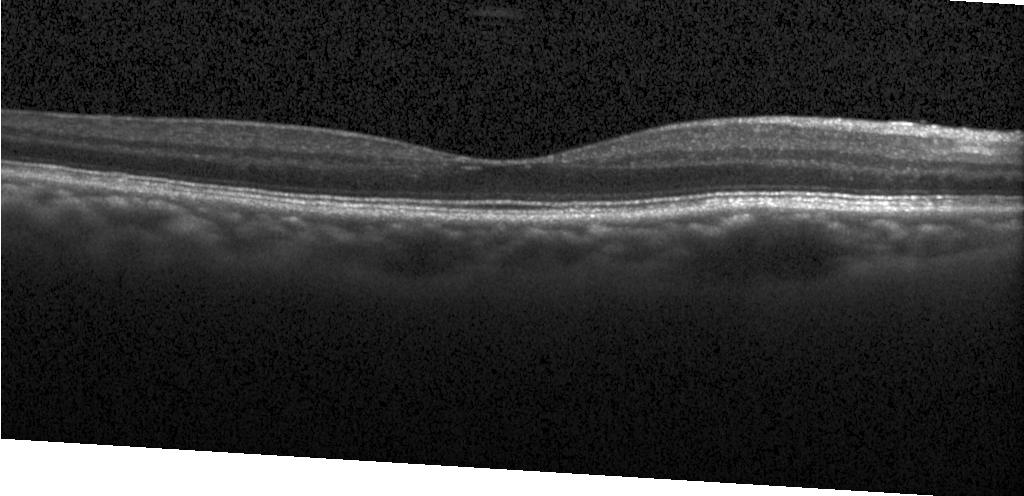
This B-scan demonstrates no choroidal neovascularization, no diabetic macular edema, and no drusen.